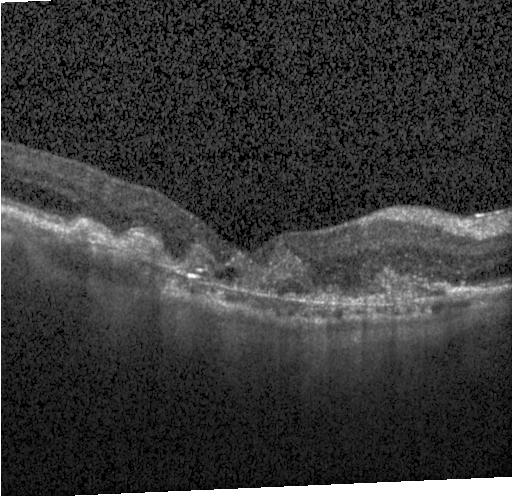 A choroidal neovascular membrane.